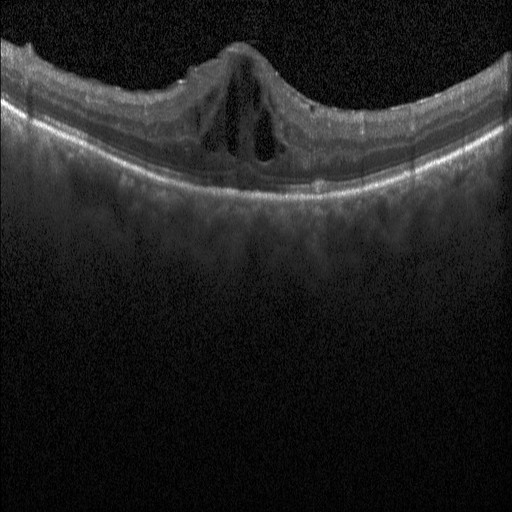 Diagnosis: diabetic macular edema (DME).